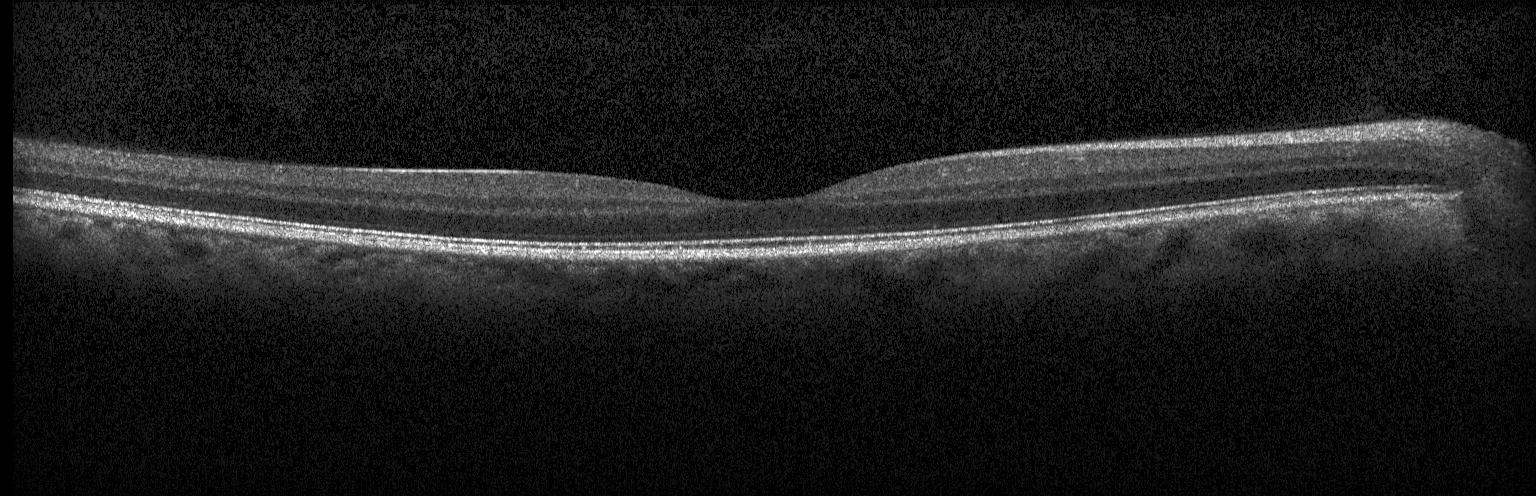 Macular OCT demonstrating neither choroidal neovascularization, diabetic macular edema, nor drusen.